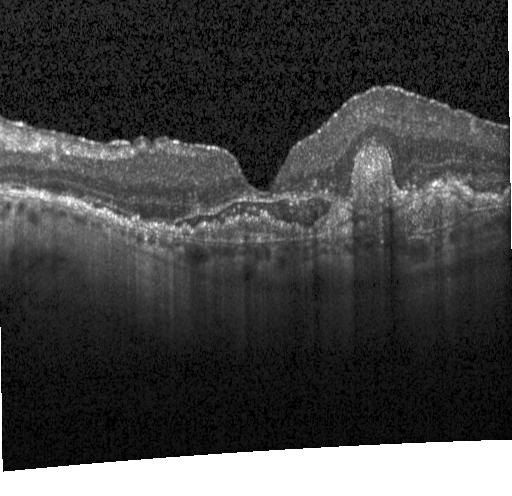

Finding: a choroidal neovascular membrane.